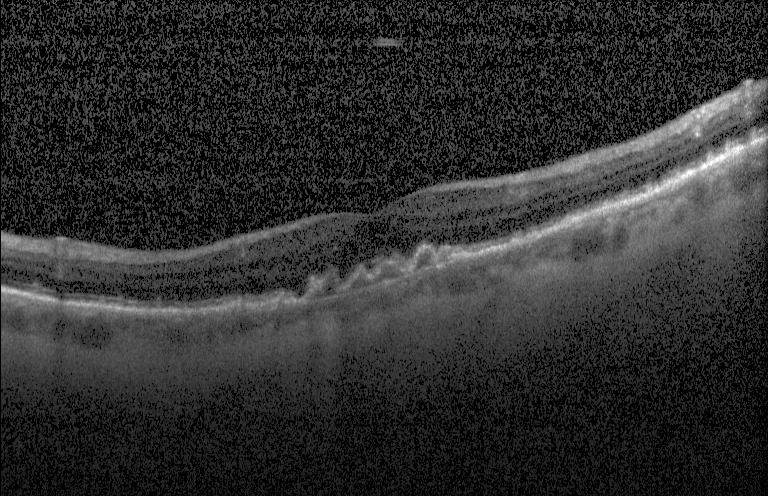

Retinal OCT cross-section showing a choroidal neovascular membrane.